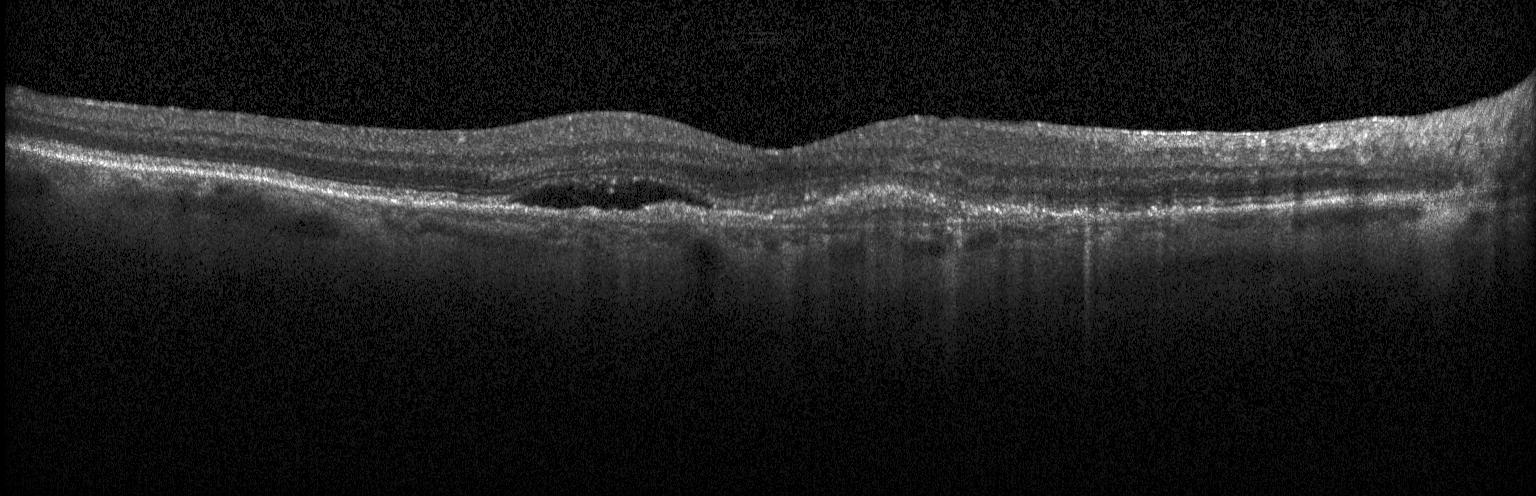
Retinal OCT cross-section; SD-OCT; Heidelberg Spectralis.
Finding: choroidal neovascularization.